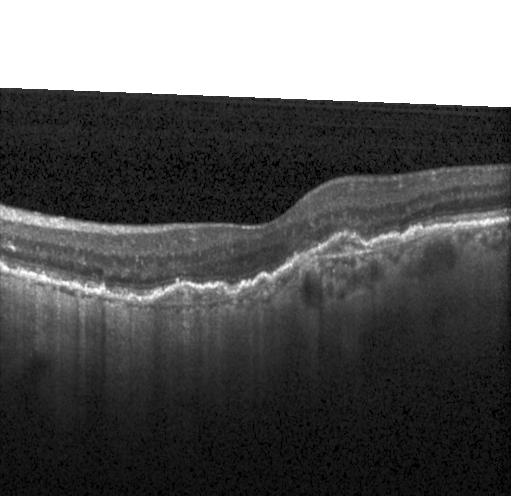

Retinal OCT B-scan — This B-scan demonstrates a choroidal neovascular membrane.